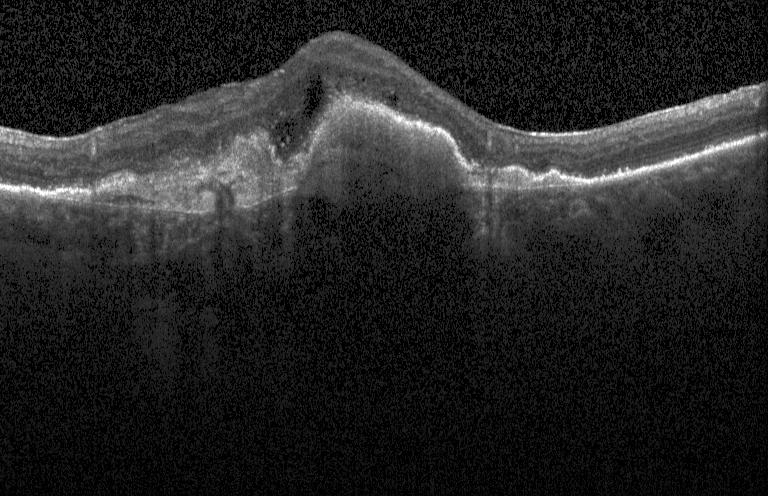
Macular scan. OCT line scan. Heidelberg Spectralis.
This B-scan demonstrates a choroidal neovascular membrane.